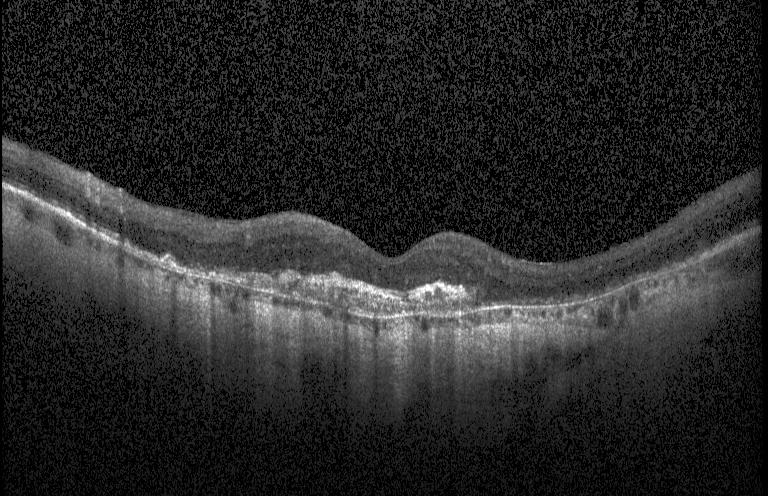
Assessment: CNV.